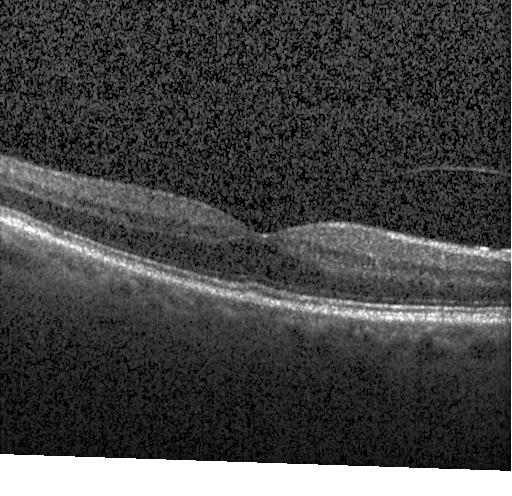
Horizontal scan through the fovea · retinal OCT B-scan · SD-OCT.
Impression: no choroidal neovascularization, diabetic macular edema, or drusen.